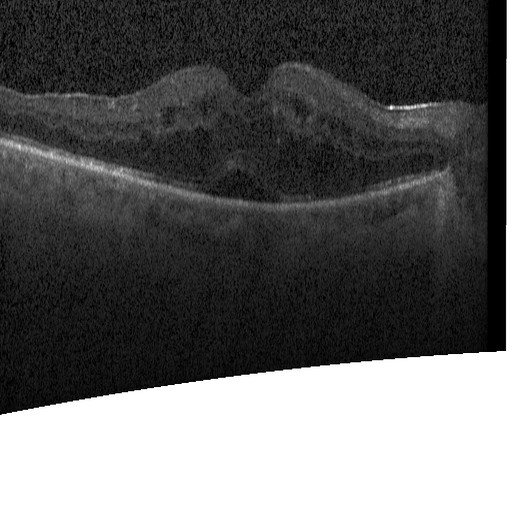 OCT B-scan. Acquired on a Heidelberg Spectralis.
Impression: DME.